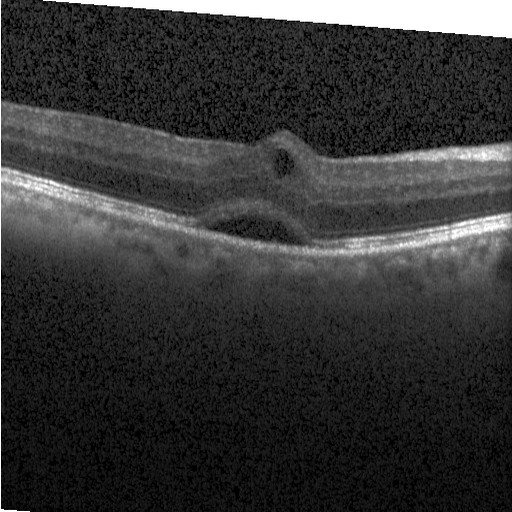

OCT B-scan showing diabetic macular edema (DME).